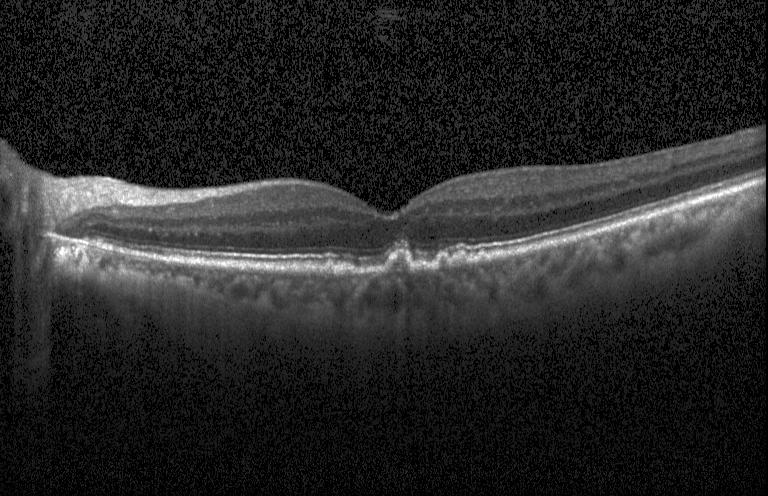

Centered on the fovea. Heidelberg Spectralis OCT system. Spectral-domain optical coherence tomography. Retinal OCT cross-section.
Macular OCT: sub-RPE drusenoid deposits.